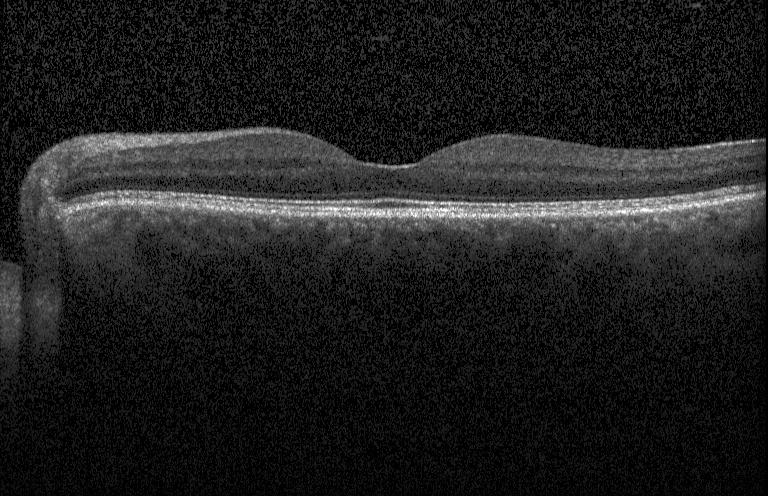
Optical coherence tomography scan. Heidelberg Spectralis. Fovea-centered. Assessment: no evidence of choroidal neovascularization, diabetic macular edema, or drusen.